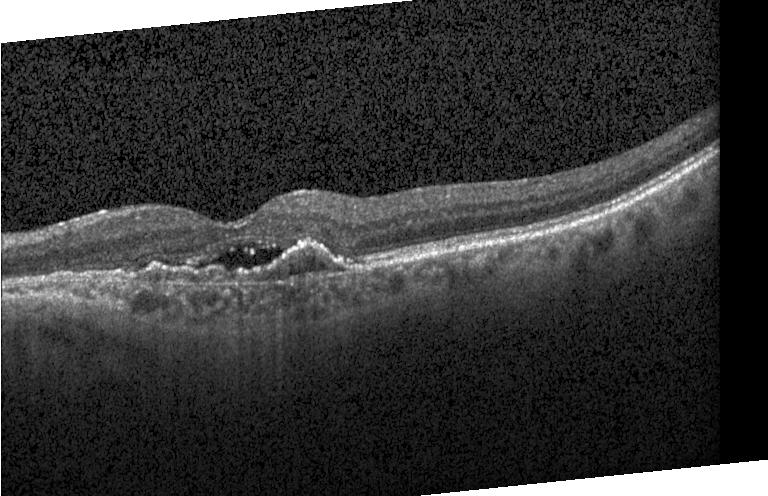

OCT B-scan. Through the macula.
Diagnosis: a choroidal neovascular membrane.